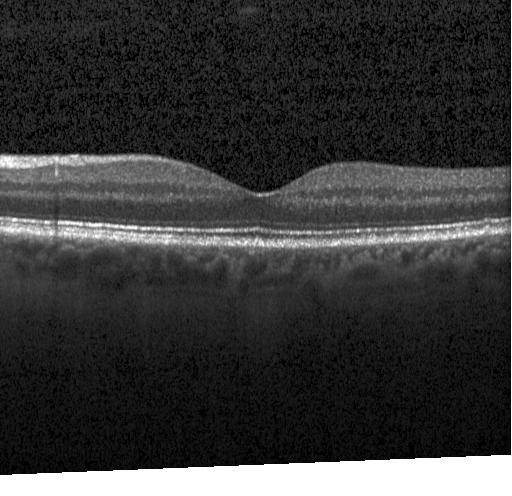
Diagnosis: no choroidal neovascularization, no diabetic macular edema, and no drusen.